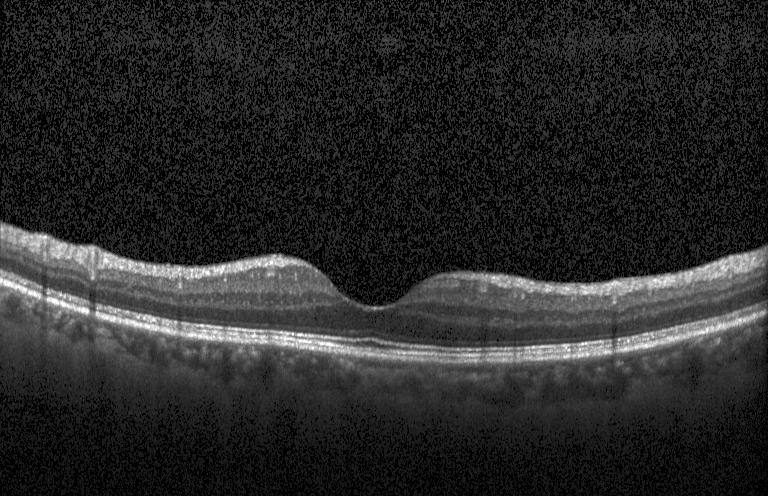
Fovea-centered; Heidelberg Spectralis; optical coherence tomography B-scan
Dx: no evidence of choroidal neovascularization, diabetic macular edema, or drusen.